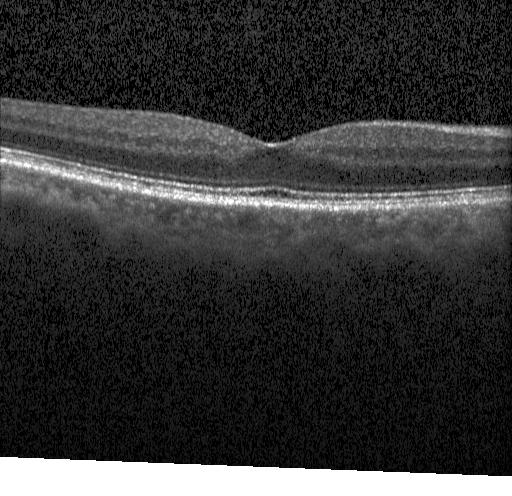
Retinal OCT B-scan, spectral-domain OCT, macular scan.
Dx: no evidence of choroidal neovascularization, diabetic macular edema, or drusen.